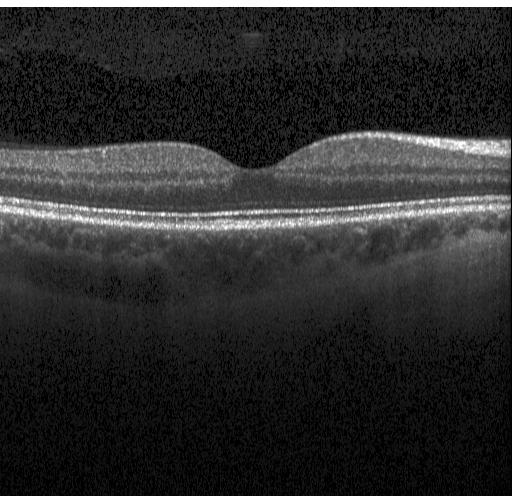
Retinal OCT B-scan
Diagnosis: no choroidal neovascularization, diabetic macular edema, or drusen.